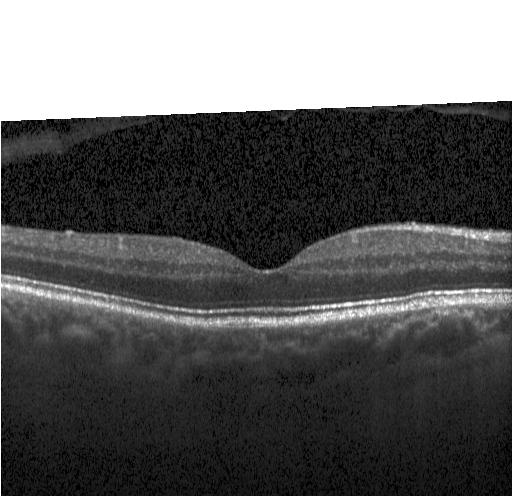
Spectral-domain OCT. OCT line scan. Through the macula.
The scan shows no choroidal neovascularization, diabetic macular edema, or drusen.